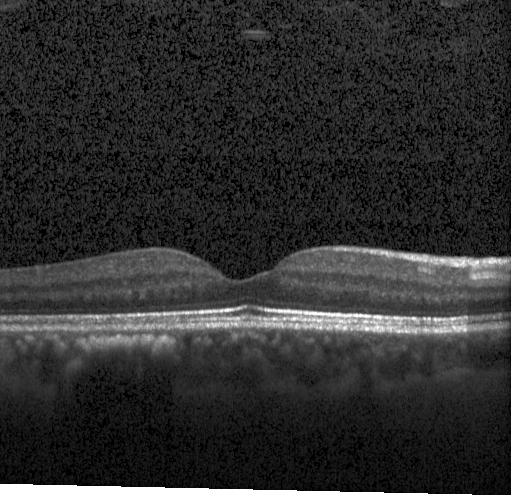
OCT B-scan · instrument: Heidelberg Spectralis — Diagnosis: no evidence of choroidal neovascularization, diabetic macular edema, or drusen.